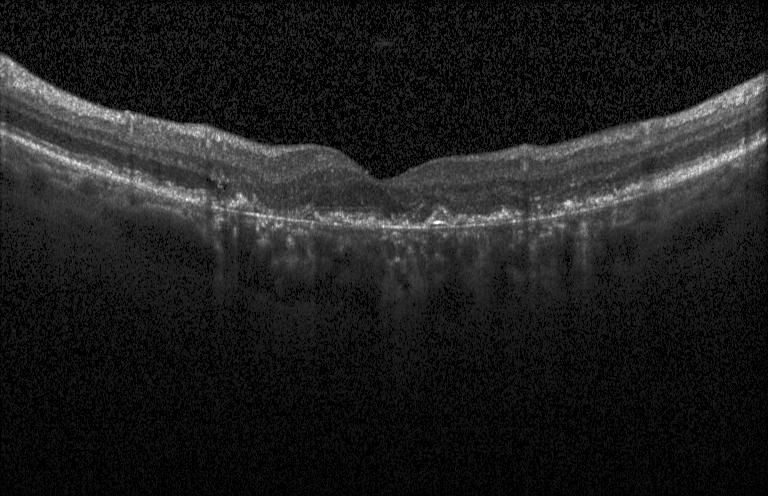

Retinal OCT cross-section
Impression: a choroidal neovascular membrane.